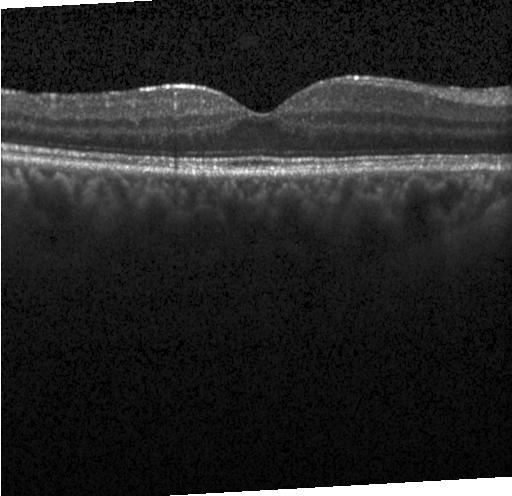
Optical coherence tomography scan · spectral-domain OCT · horizontal scan through the fovea — Impression: no CNV, DME, or drusen.